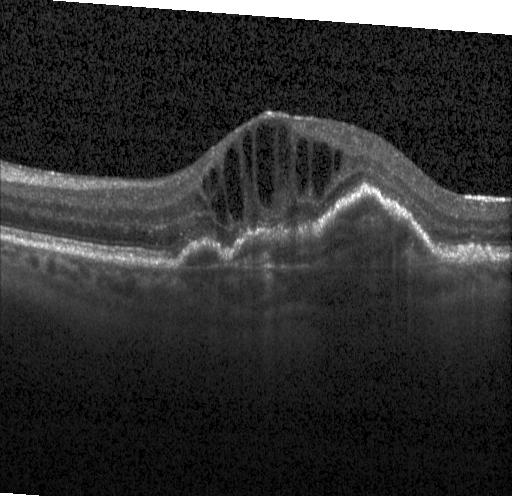 Optical coherence tomography scan. Spectral-domain optical coherence tomography. Fovea-centered. Heidelberg Spectralis OCT system
Choroidal neovascularization (CNV).